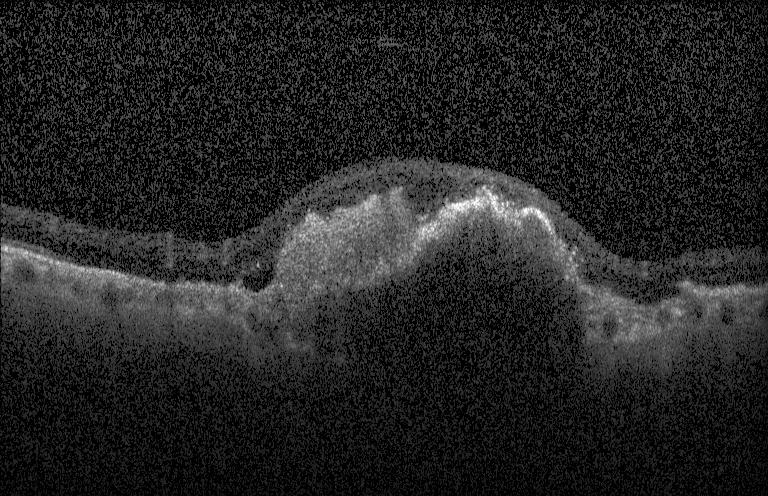 Centered on the fovea, Heidelberg Spectralis OCT system, OCT B-scan, spectral-domain optical coherence tomography — Finding: a choroidal neovascular membrane.